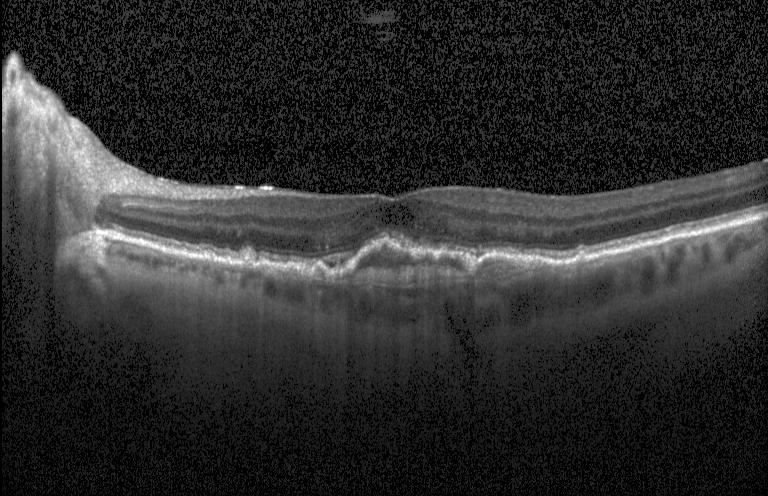 Fovea-centered, OCT line scan, spectral-domain OCT. A choroidal neovascular membrane.